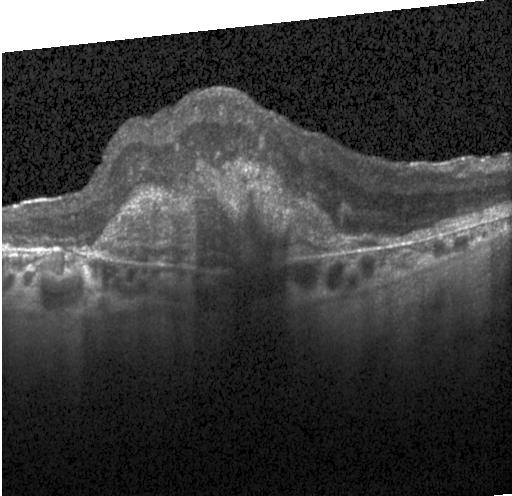
Impression: choroidal neovascularization (CNV).